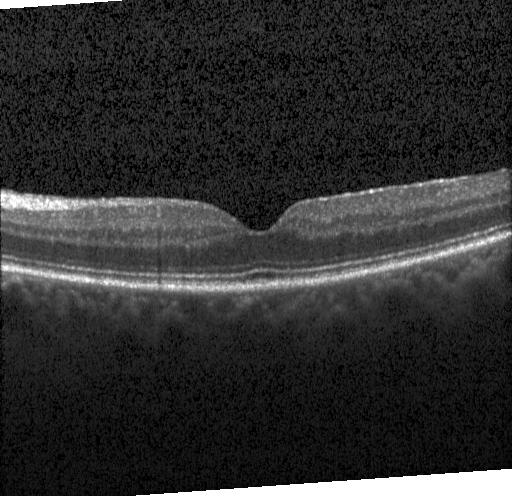 Spectral-domain optical coherence tomography, macular scan, Heidelberg Spectralis, optical coherence tomography B-scan. Impression: no evidence of choroidal neovascularization, diabetic macular edema, or drusen.